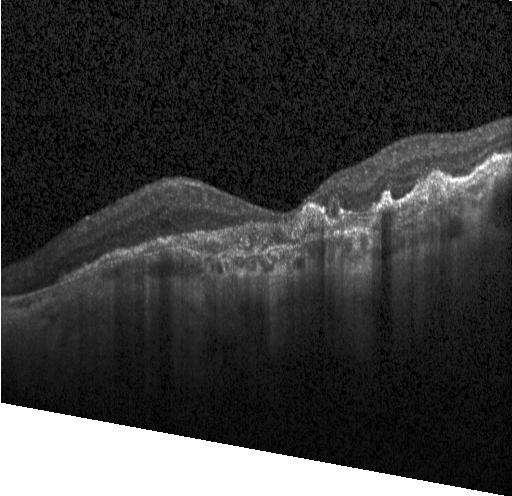

Centered on the fovea; optical coherence tomography scan; acquired on a Heidelberg Spectralis; SD-OCT
Diagnosis: a choroidal neovascular membrane.